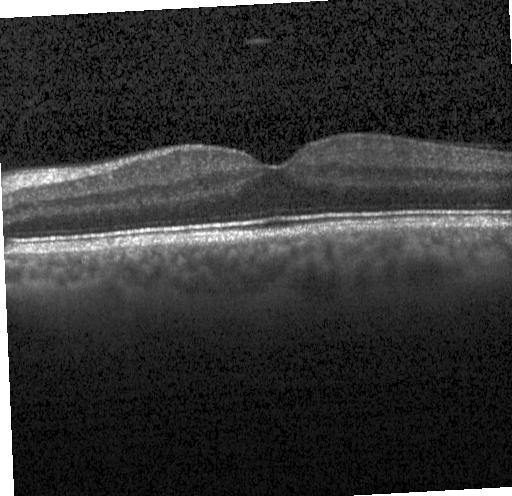 Retinal OCT B-scan; spectral-domain optical coherence tomography; fovea-centered; instrument: Heidelberg Spectralis.
Finding: no CNV, DME, or drusen.